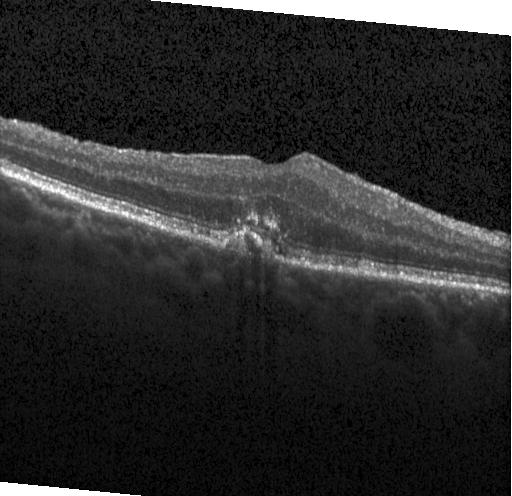

Instrument: Heidelberg Spectralis; spectral-domain OCT; retinal OCT cross-section; horizontal scan through the fovea. Impression: choroidal neovascularization (CNV).